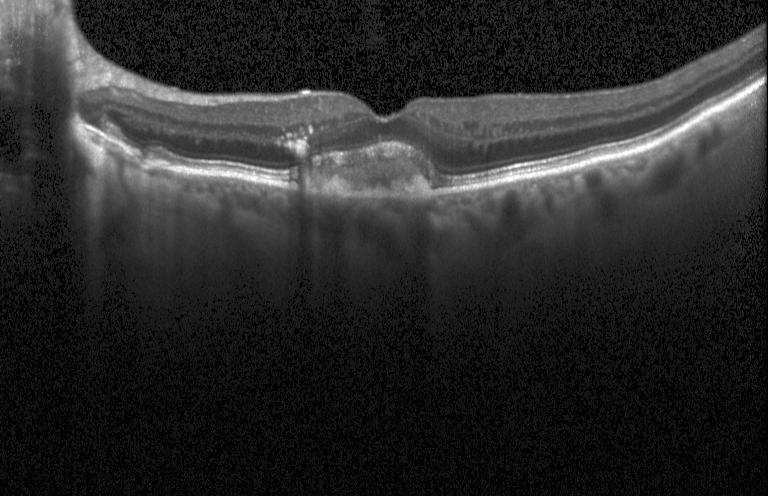 Spectral-domain OCT B-scan: choroidal neovascularization.